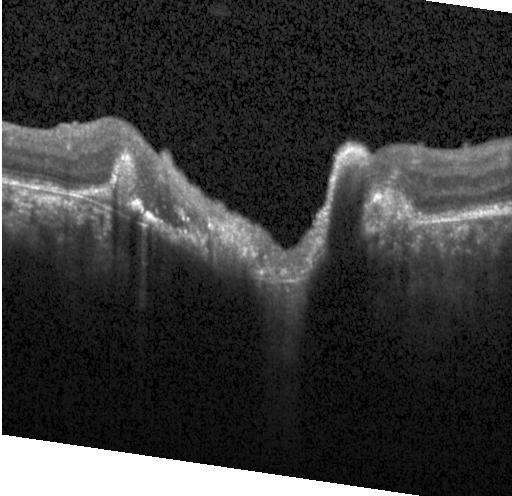 OCT line scan. Diagnosis: choroidal neovascularization (CNV).